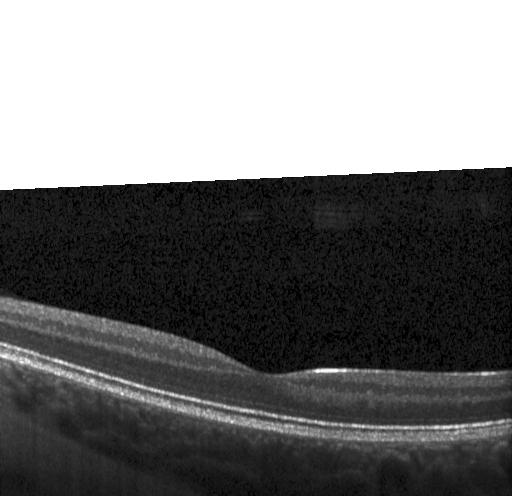

OCT B-scan.
Assessment: neither choroidal neovascularization, diabetic macular edema, nor drusen.